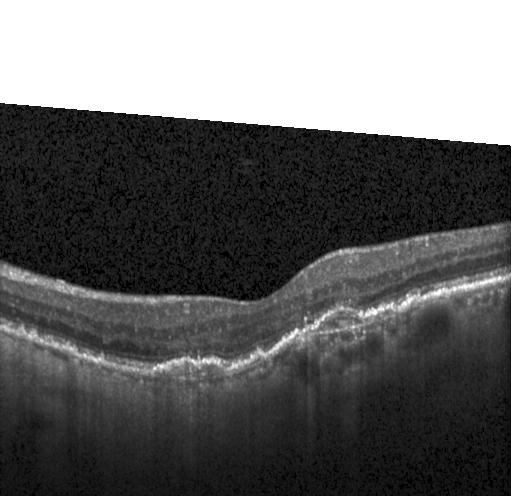 Impression: CNV.